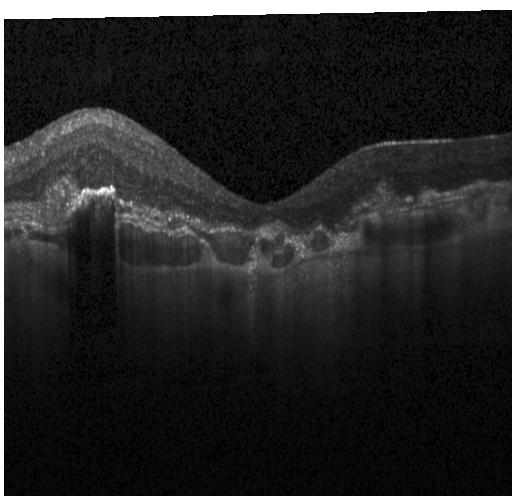
SD-OCT · retinal OCT B-scan
Dx: choroidal neovascularization (CNV).